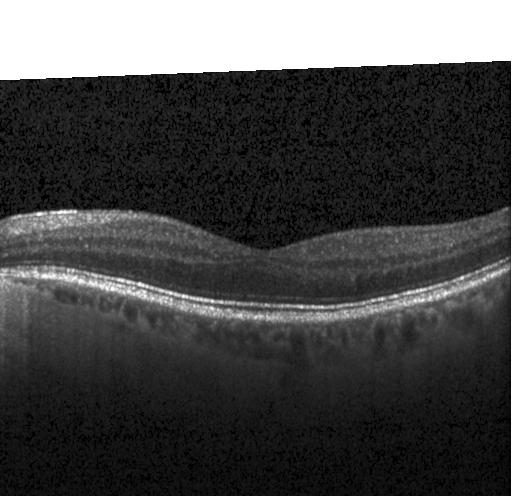
Dx: no evidence of CNV, DME, or drusen.